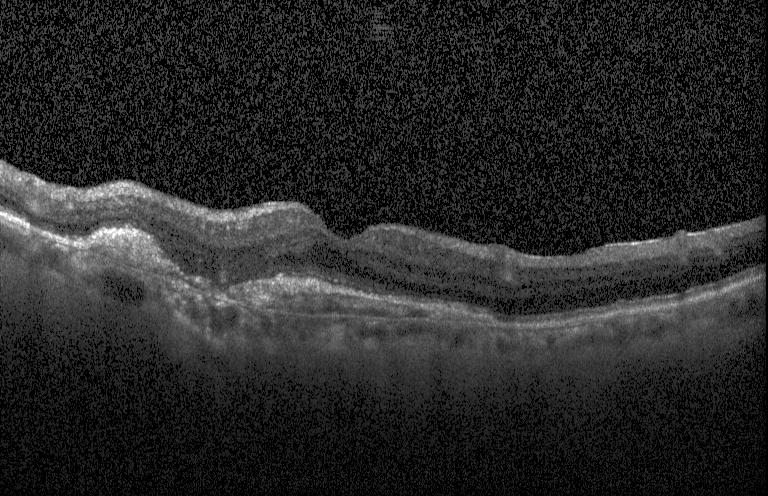

OCT finding: a choroidal neovascular membrane.